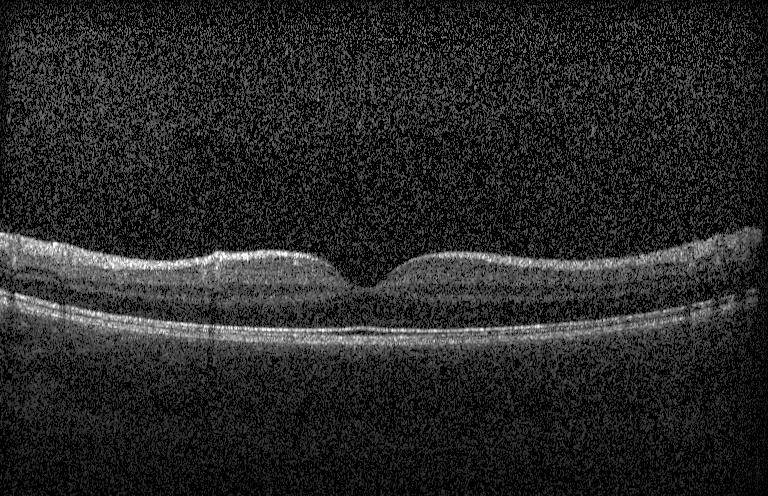 Impression: no choroidal neovascularization, no diabetic macular edema, and no drusen.